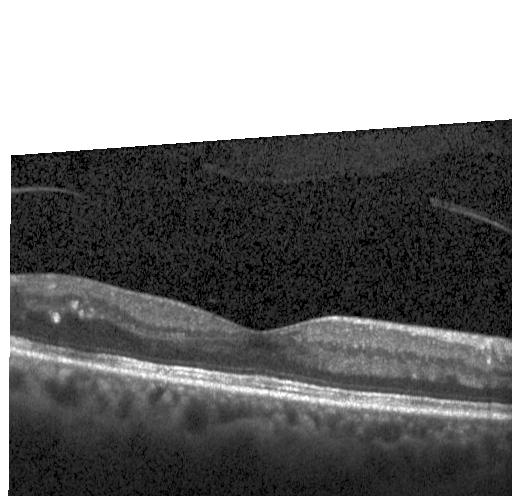

Through the macula. Acquired on a Heidelberg Spectralis. Spectral-domain OCT. OCT B-scan — Impression: DME.